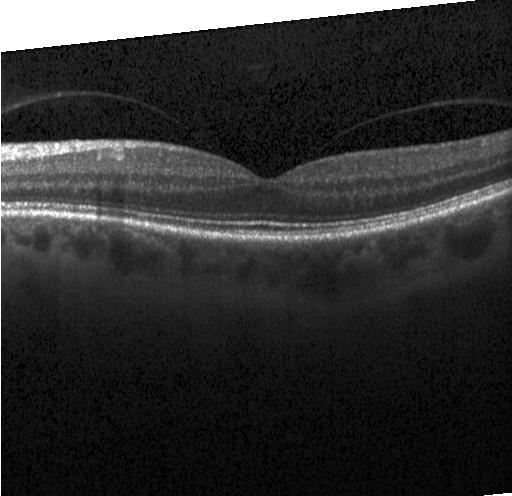
Macular OCT: neither choroidal neovascularization, diabetic macular edema, nor drusen.